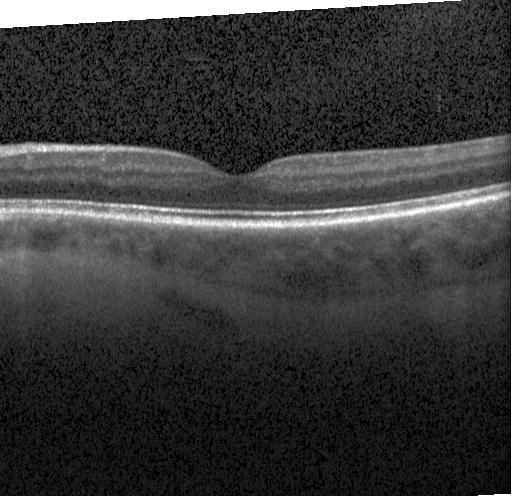

Macular OCT: no CNV, DME, or drusen.